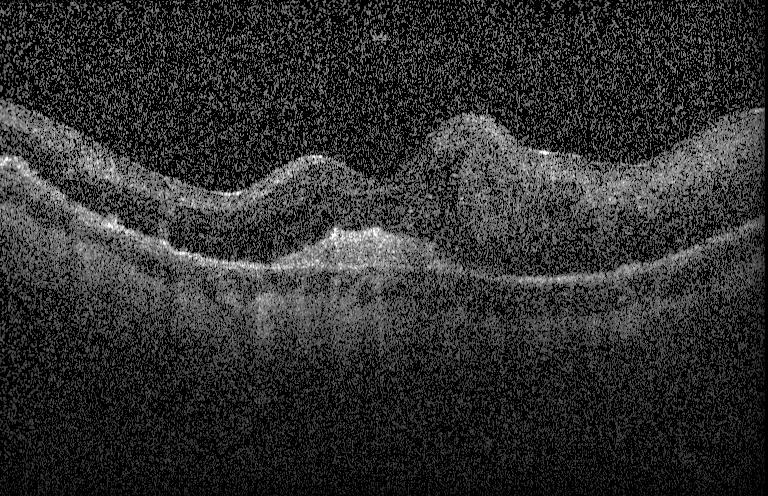
Optical coherence tomography B-scan. Macular scan. Heidelberg Spectralis — This B-scan demonstrates a choroidal neovascular membrane.